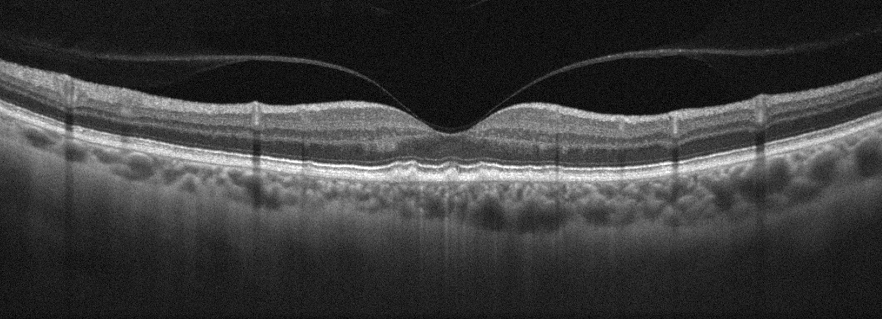
Through the macula. OCT line scan. Instrument: Optovue Avanti RTVue XR — The scan shows age-related macular degeneration (AMD).